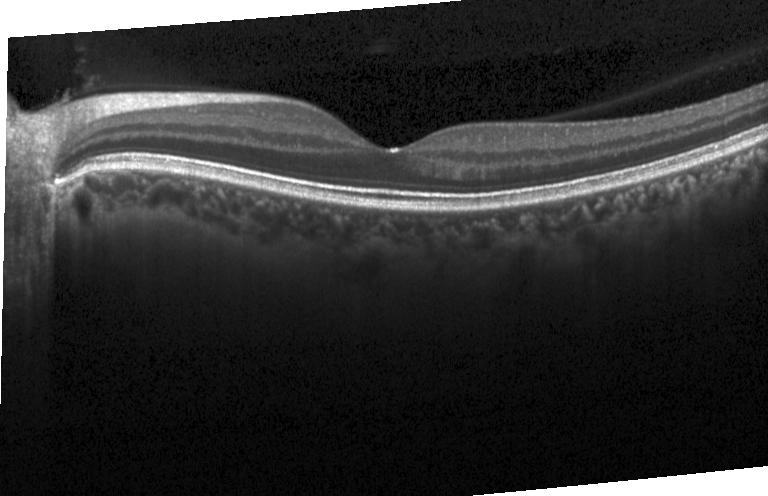 Finding: no evidence of choroidal neovascularization, diabetic macular edema, or drusen.